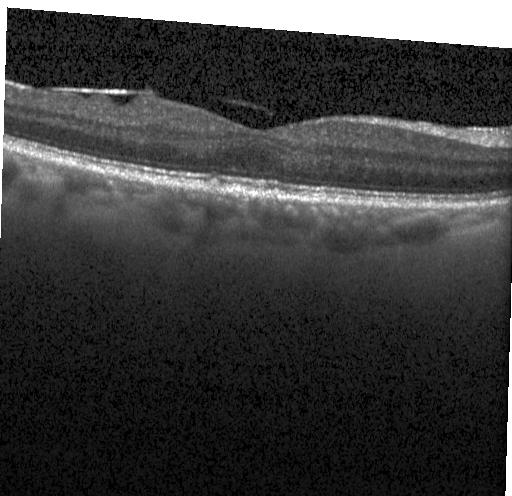

OCT line scan. Finding: multiple drusen.